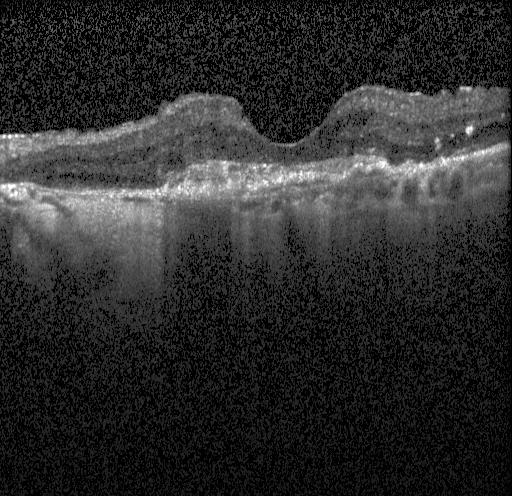

Impression: a choroidal neovascular membrane.